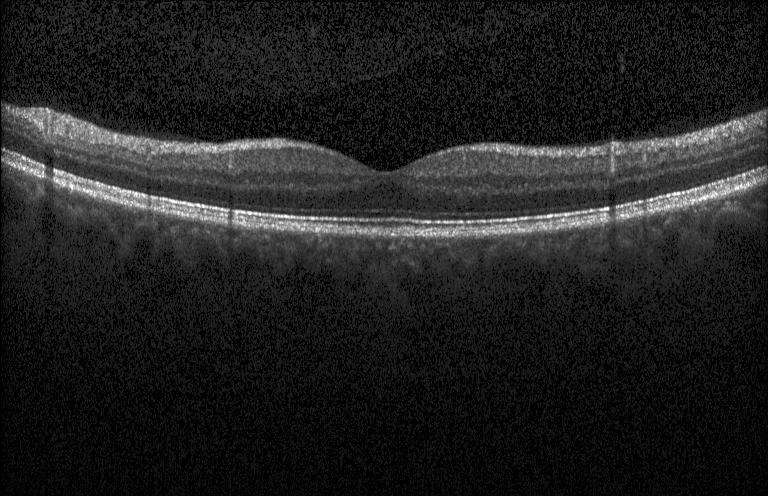

Fovea-centered, OCT line scan, spectral-domain OCT, Heidelberg Spectralis OCT system — This B-scan demonstrates neither choroidal neovascularization, diabetic macular edema, nor drusen.